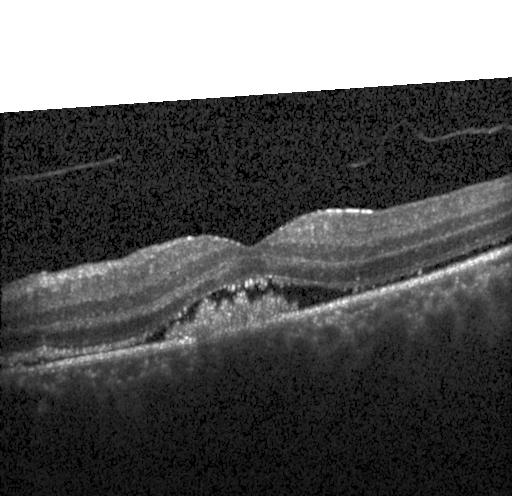
Macular OCT: choroidal neovascularization.